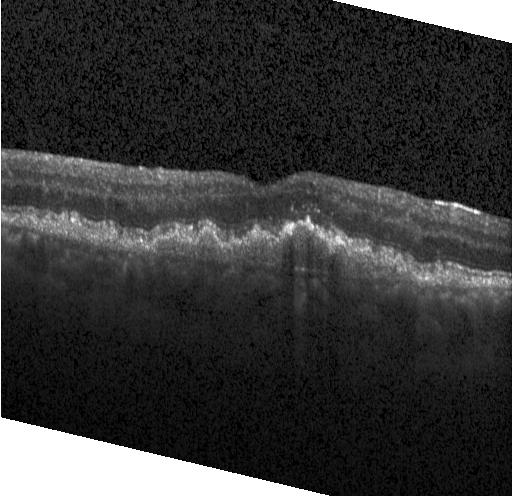

Retinal OCT cross-section
This B-scan demonstrates a choroidal neovascular membrane.